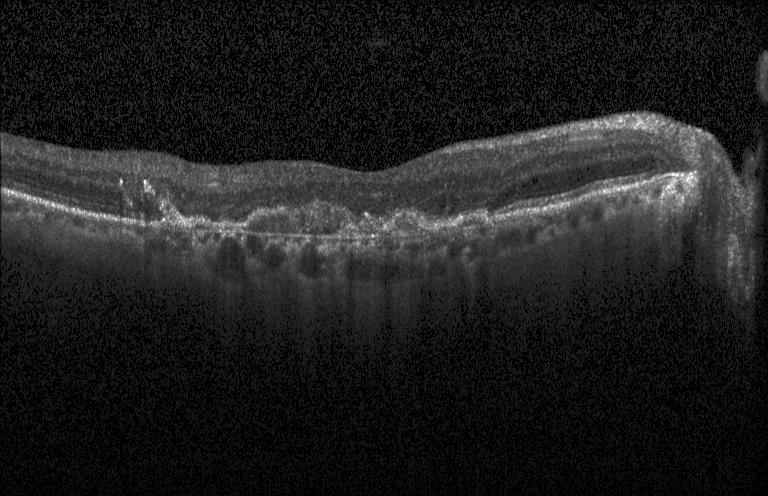 A choroidal neovascular membrane.